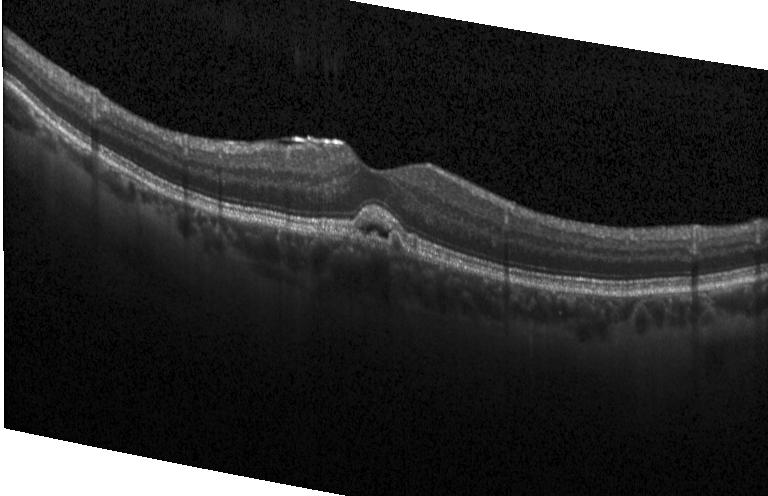

Retinal OCT B-scan; macular scan.
Finding: choroidal neovascularization (CNV).